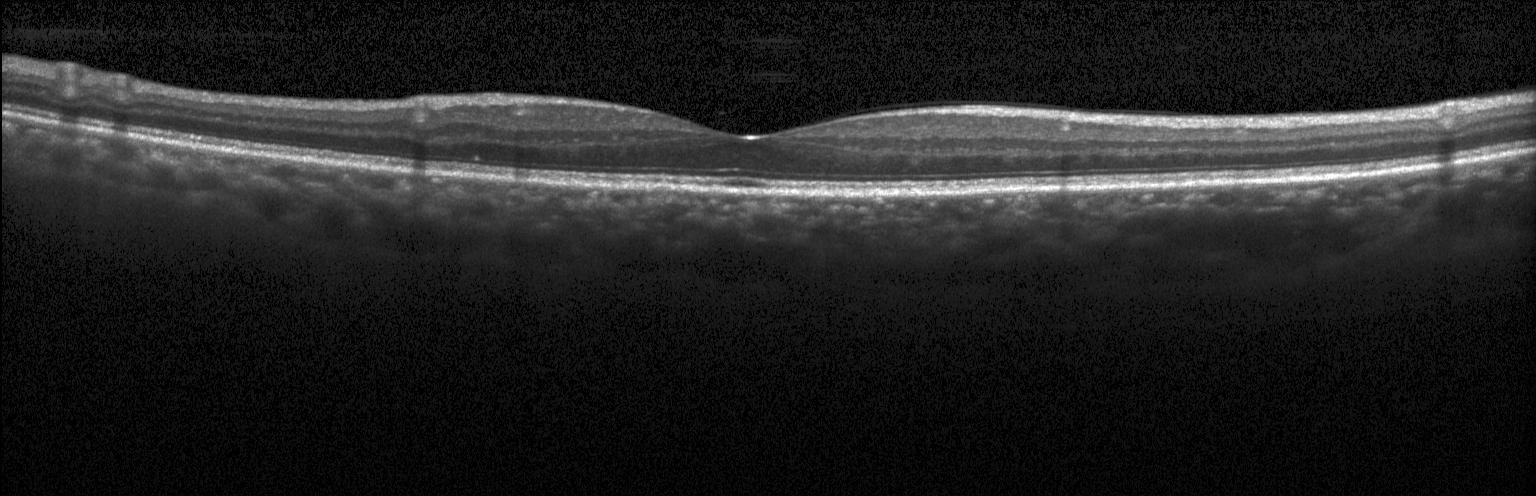

OCT scan showing no choroidal neovascularization, no diabetic macular edema, and no drusen.